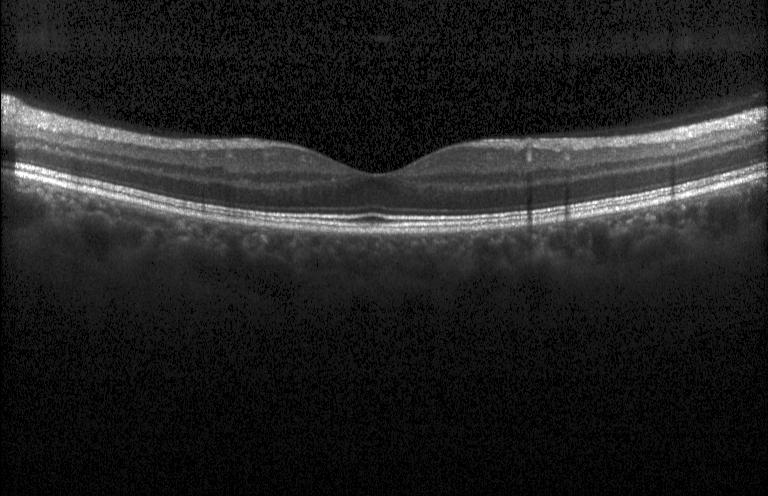

This B-scan demonstrates neither CNV, DME, nor drusen.